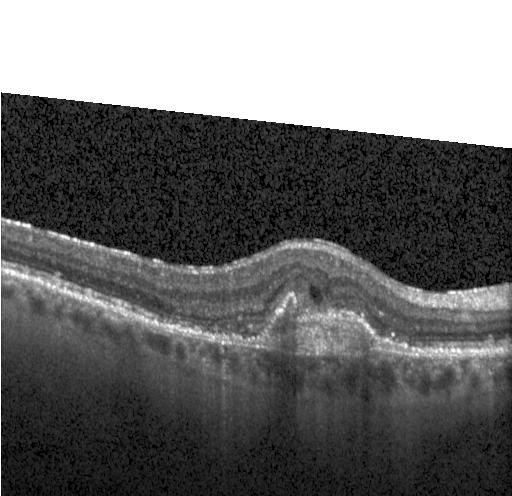
The scan shows choroidal neovascularization (CNV).